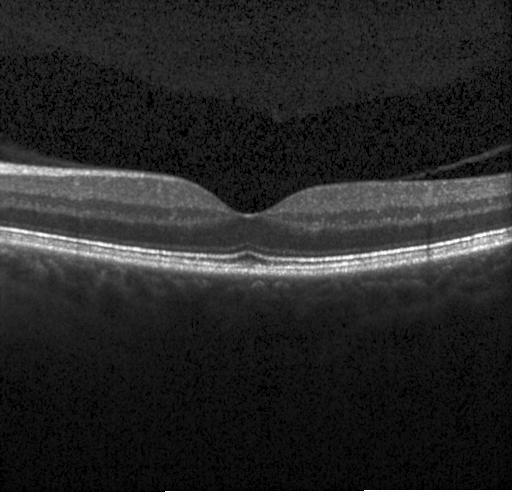
This B-scan demonstrates no CNV, no DME, and no drusen.